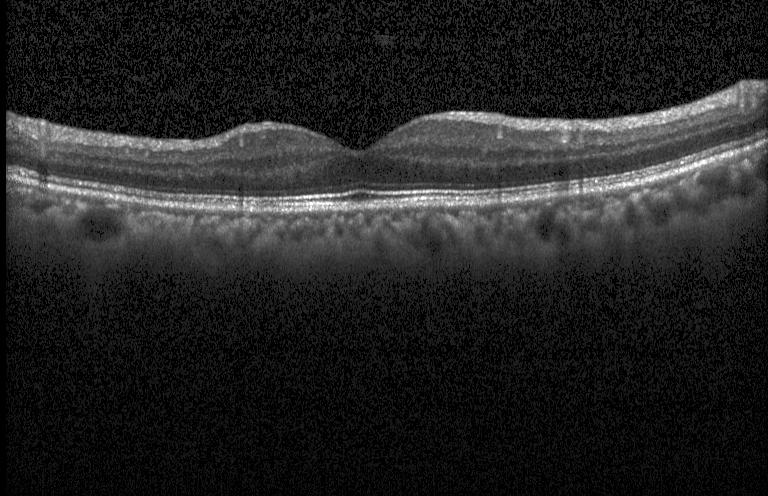
OCT B-scan · through the macula · instrument: Heidelberg Spectralis. Assessment: neither CNV, DME, nor drusen.